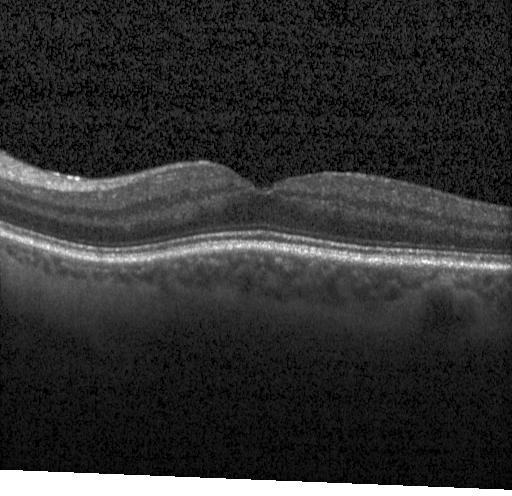

Impression: neither CNV, DME, nor drusen.